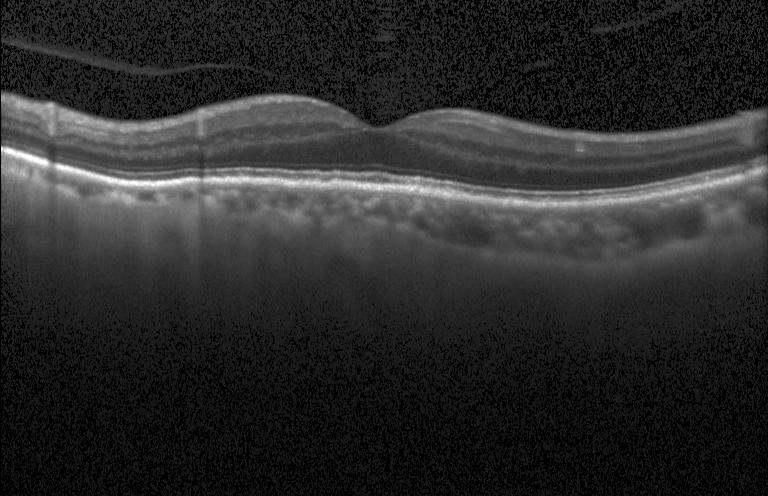
Macular scan · retinal OCT B-scan — Finding: no evidence of choroidal neovascularization, diabetic macular edema, or drusen.